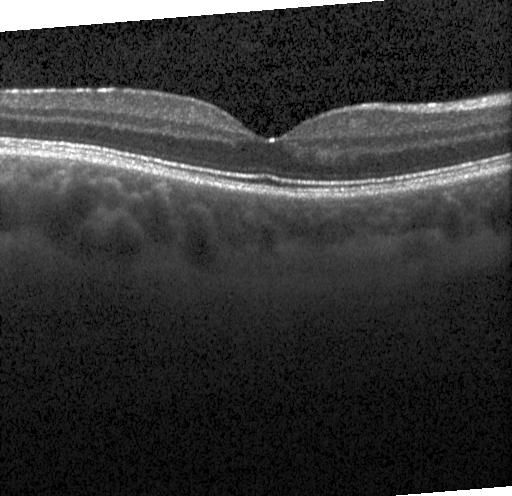

Heidelberg Spectralis. Spectral-domain optical coherence tomography. OCT line scan.
Diagnosis: neither choroidal neovascularization, diabetic macular edema, nor drusen.